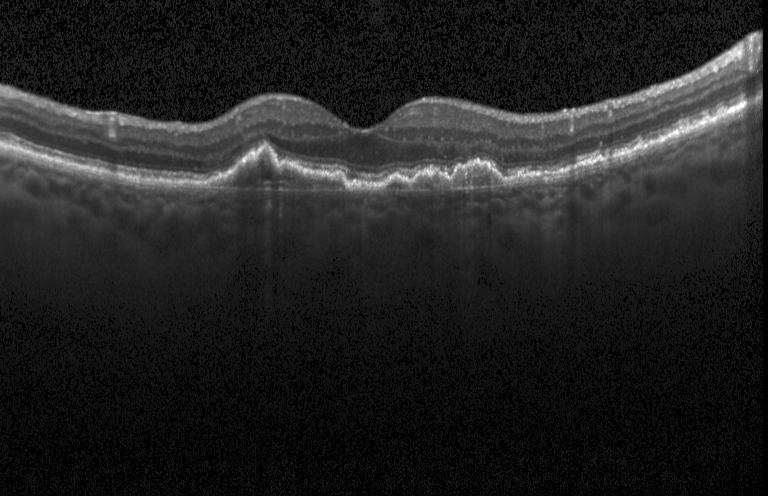 Diagnosis: a choroidal neovascular membrane.